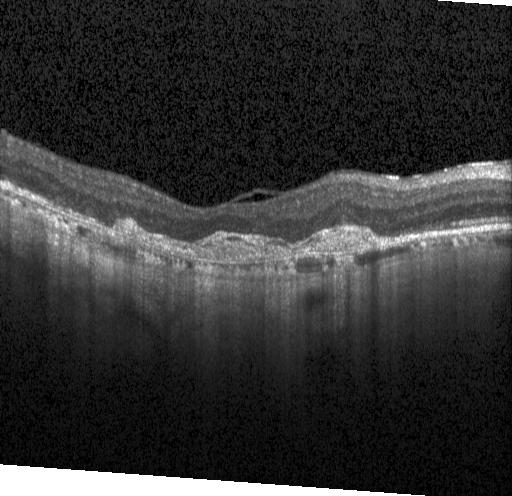
Optical coherence tomography B-scan, macular scan, SD-OCT, Heidelberg Spectralis OCT system. This B-scan demonstrates a choroidal neovascular membrane.